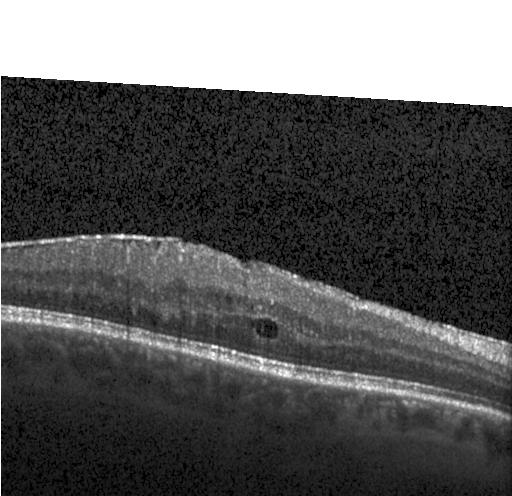

Impression: diabetic macular edema.